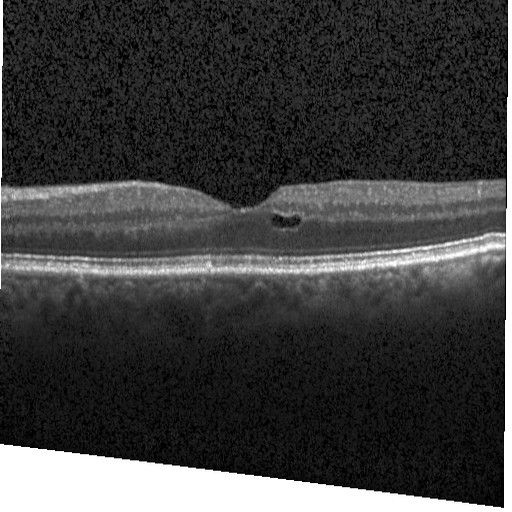 OCT line scan, instrument: Heidelberg Spectralis. Diagnosis: diabetic macular edema (DME).